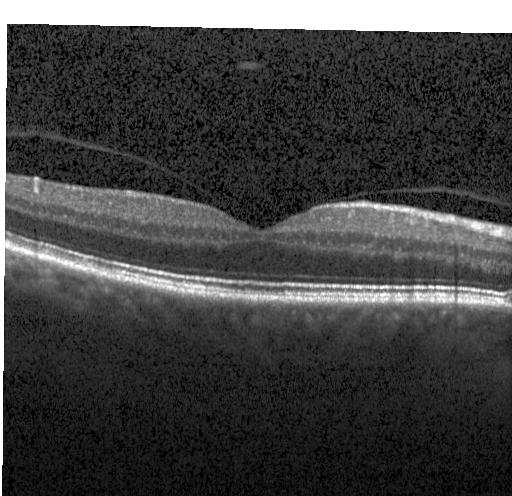
Macular scan · SD-OCT · Heidelberg Spectralis OCT system · retinal OCT cross-section — Impression: no evidence of choroidal neovascularization, diabetic macular edema, or drusen.